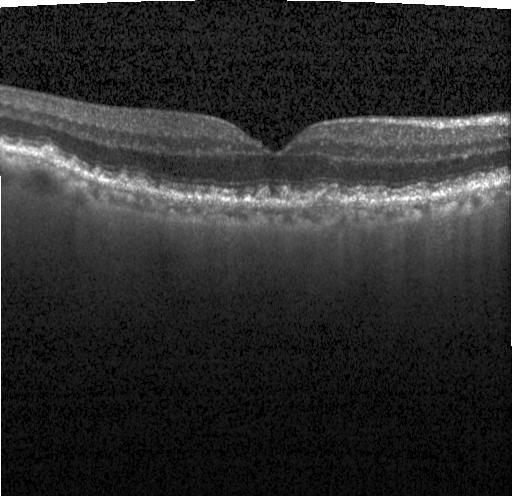

Retinal OCT cross-section. Through the macula. SD-OCT.
This B-scan demonstrates multiple drusen.